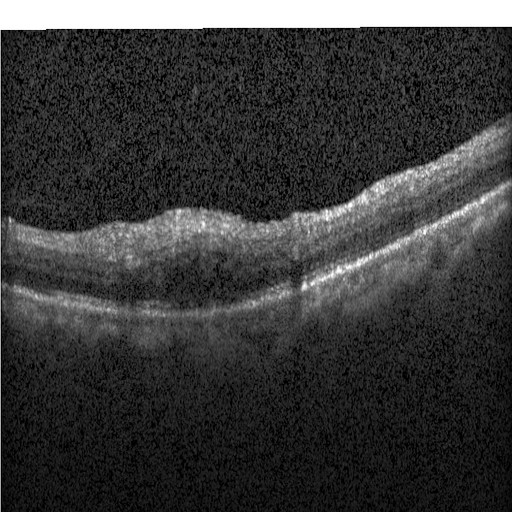 Macular OCT: diabetic macular edema.